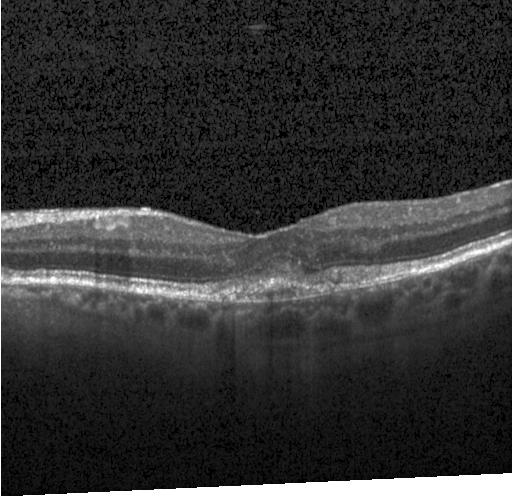
This B-scan demonstrates choroidal neovascularization (CNV).